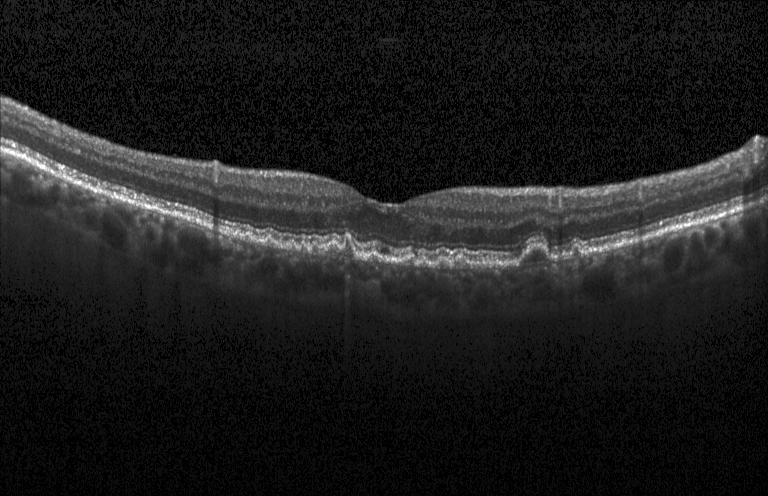

Finding: drusen.